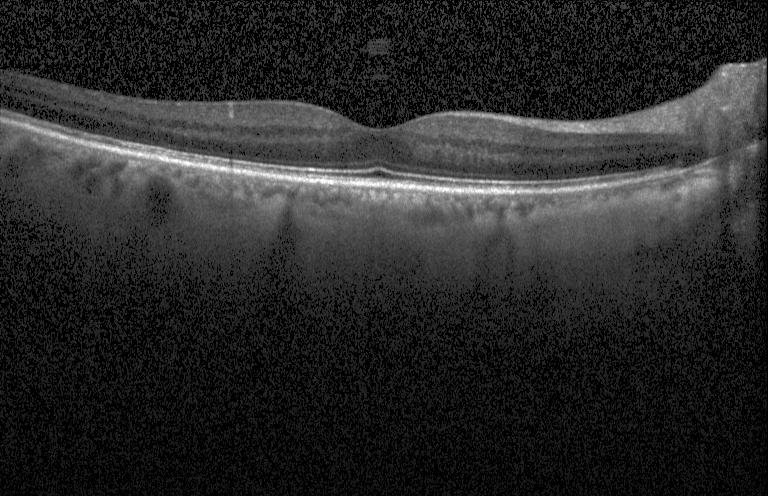
Finding: neither choroidal neovascularization, diabetic macular edema, nor drusen.